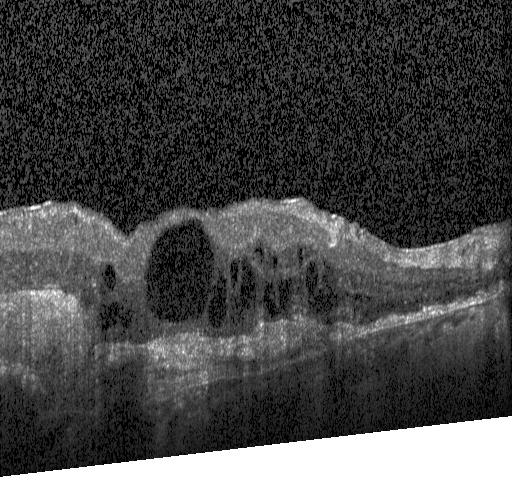
Acquired on a Heidelberg Spectralis, retinal OCT B-scan, spectral-domain OCT.
Diagnosis: choroidal neovascularization (CNV).